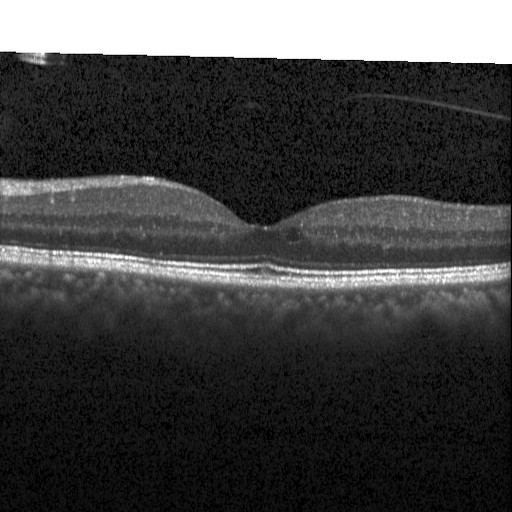 Dx: DME.